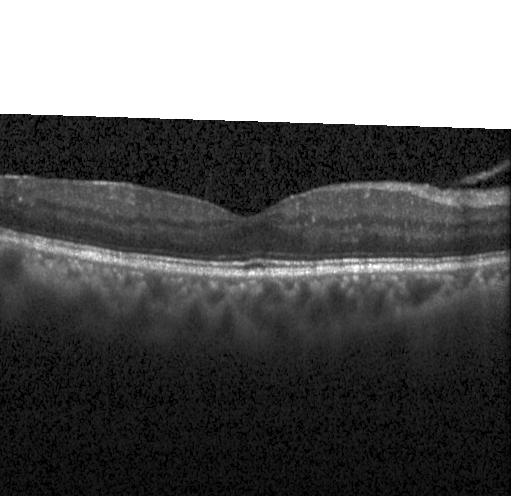
Optical coherence tomography scan. Heidelberg Spectralis OCT system. Through the macula.
Diagnosis: neither choroidal neovascularization, diabetic macular edema, nor drusen.